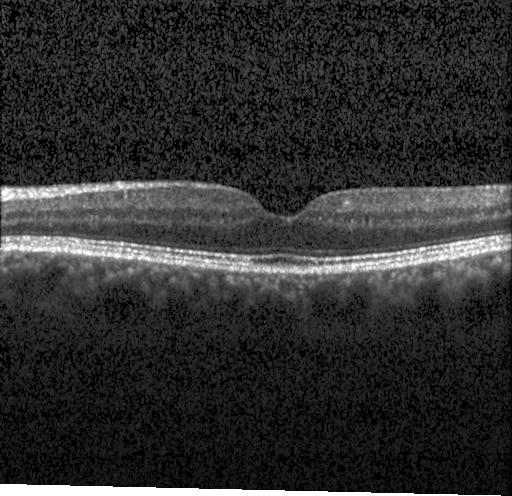

OCT B-scan showing no CNV, DME, or drusen.